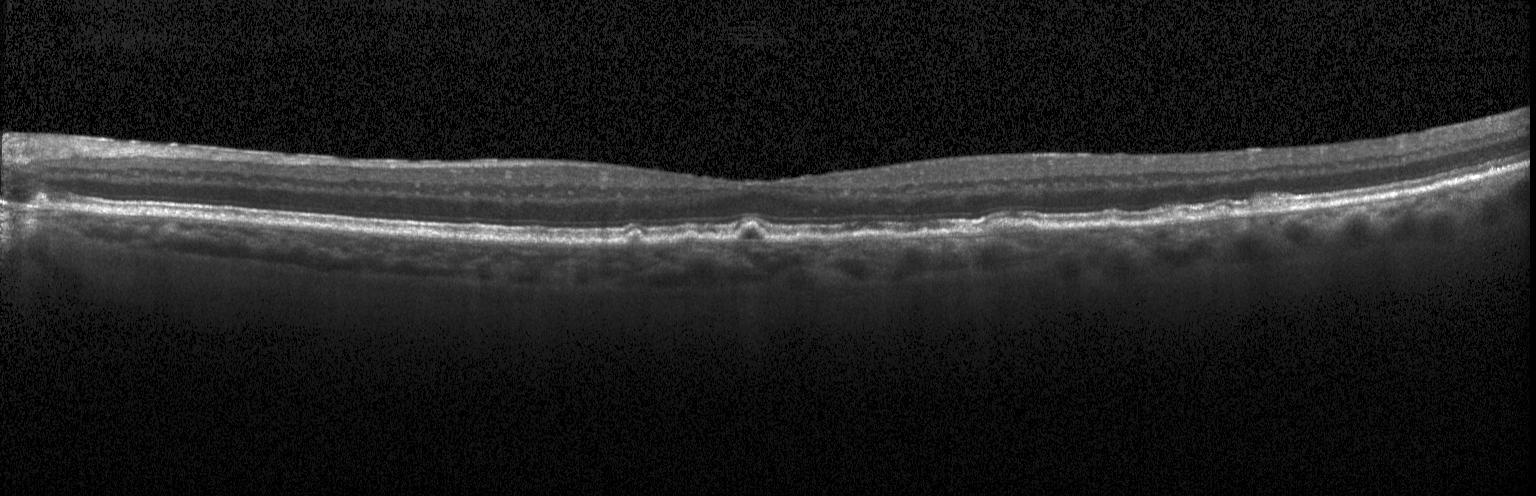
Impression: drusen.